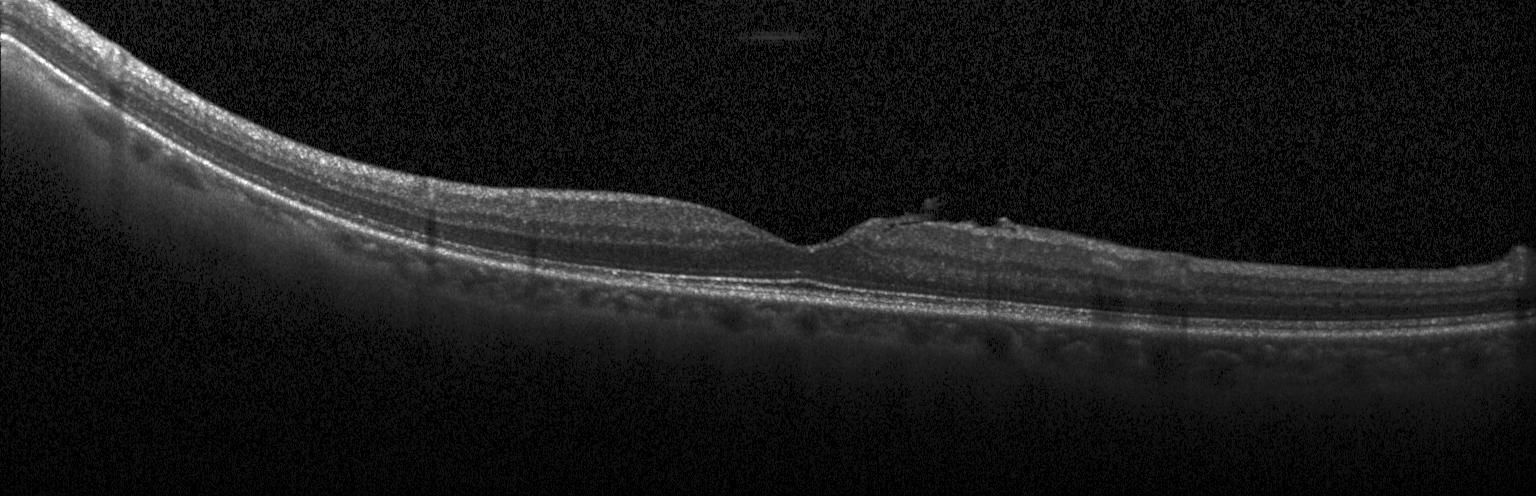
Fovea-centered; OCT line scan. Impression: no evidence of choroidal neovascularization, diabetic macular edema, or drusen.